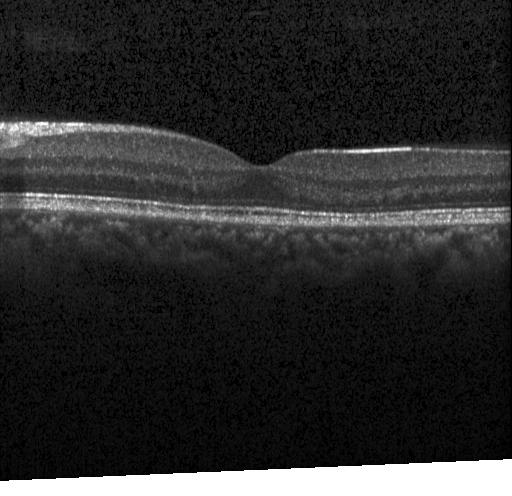

Horizontal scan through the fovea, retinal OCT B-scan, spectral-domain optical coherence tomography
Assessment: neither CNV, DME, nor drusen.